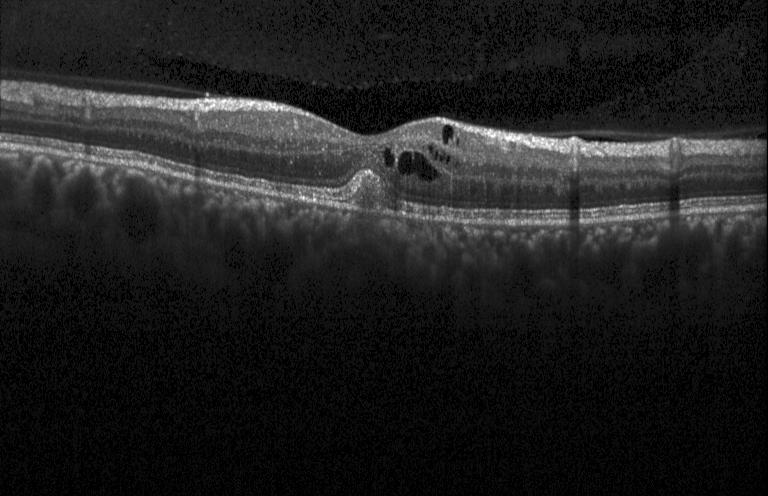

OCT B-scan showing CNV.